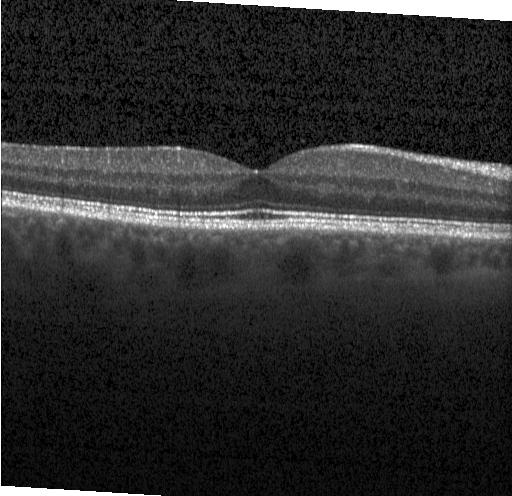

Retinal OCT B-scan. Diagnosis: no evidence of CNV, DME, or drusen.